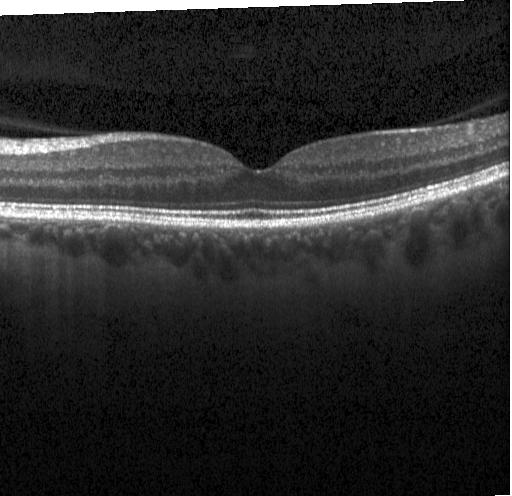
OCT B-scan showing no choroidal neovascularization, no diabetic macular edema, and no drusen.